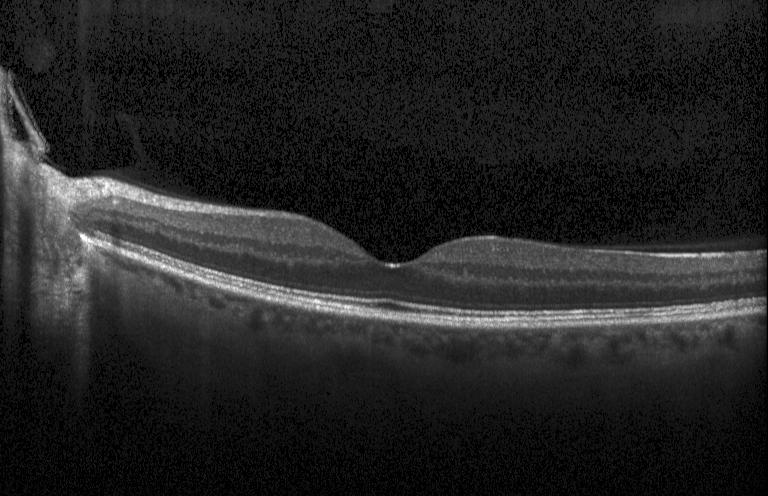
Optical coherence tomography B-scan · Heidelberg Spectralis OCT system · spectral-domain OCT · macular scan — Diagnosis: no choroidal neovascularization, no diabetic macular edema, and no drusen.